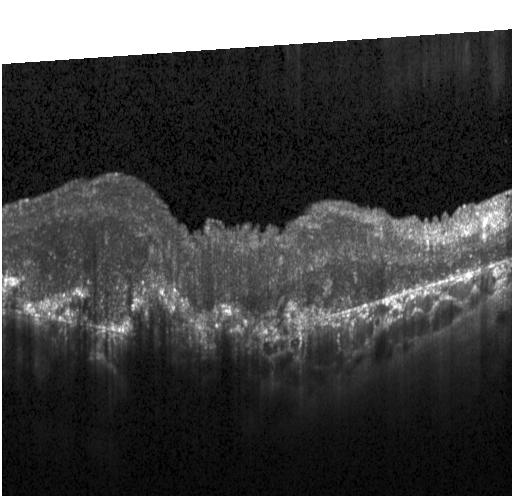 Optical coherence tomography scan
Finding: a choroidal neovascular membrane.